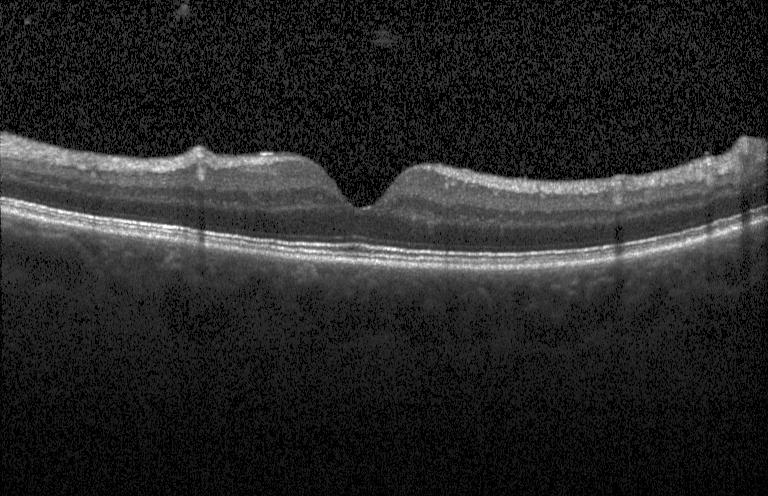 This B-scan demonstrates neither CNV, DME, nor drusen.